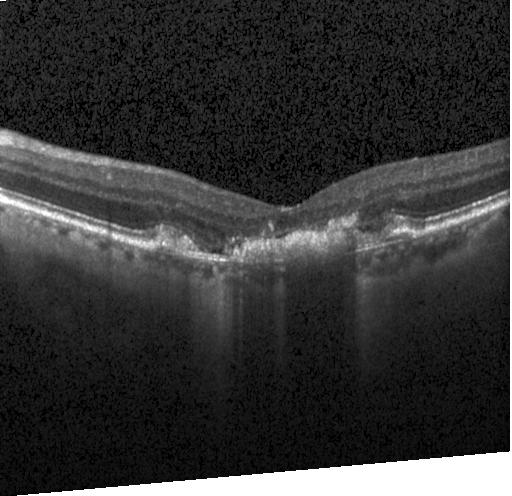

Dx: choroidal neovascularization.